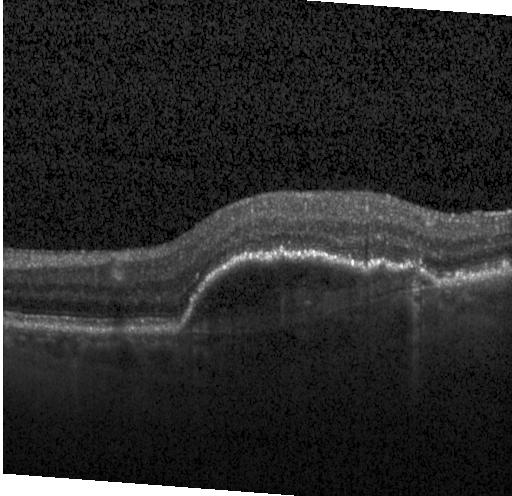 Acquired on a Heidelberg Spectralis; optical coherence tomography scan
Finding: a choroidal neovascular membrane.